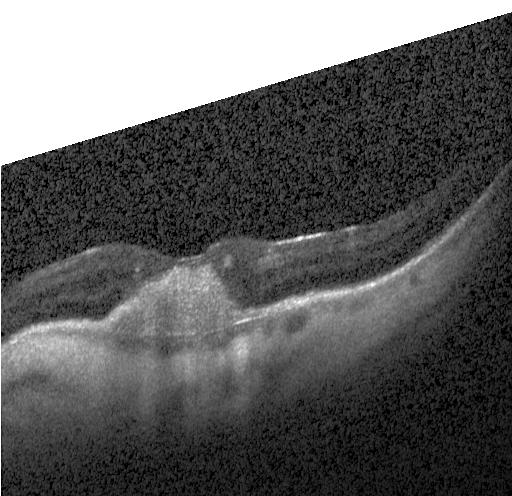
Macular OCT demonstrating choroidal neovascularization.